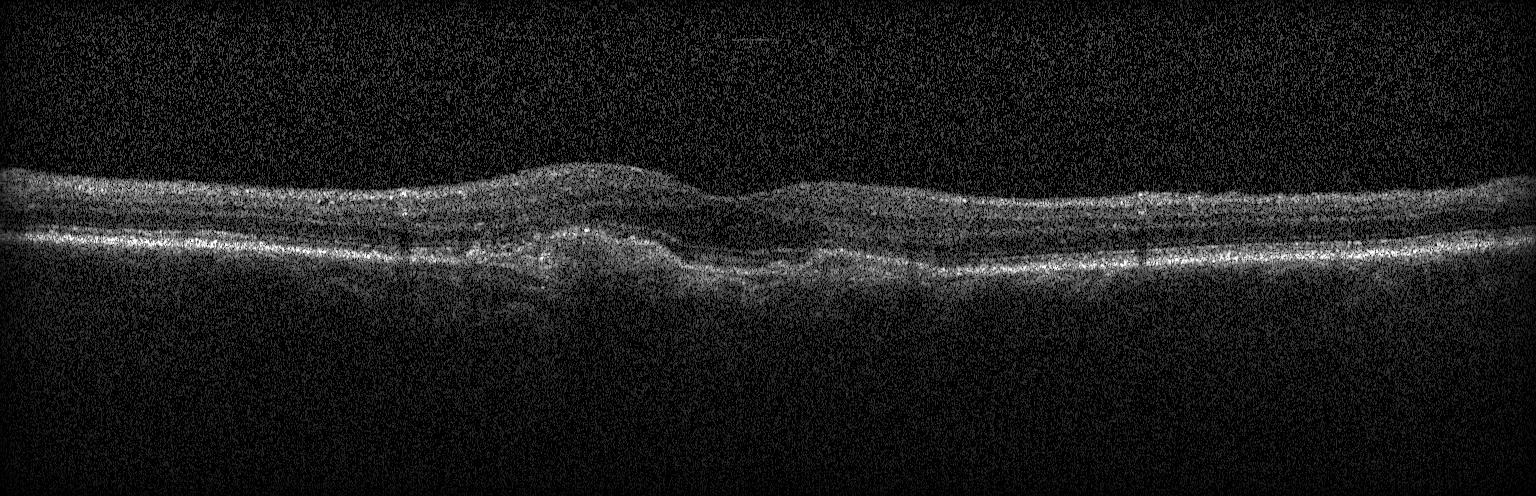

Acquired on a Heidelberg Spectralis. Retinal OCT cross-section. Horizontal scan through the fovea. Spectral-domain OCT.
Impression: choroidal neovascularization.